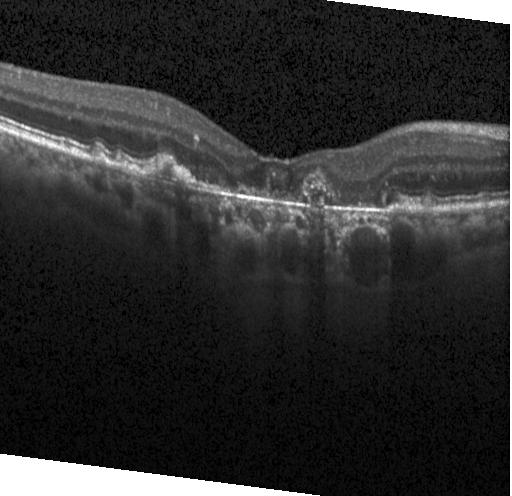

Through the macula, spectral-domain optical coherence tomography, retinal OCT B-scan. Finding: a choroidal neovascular membrane.